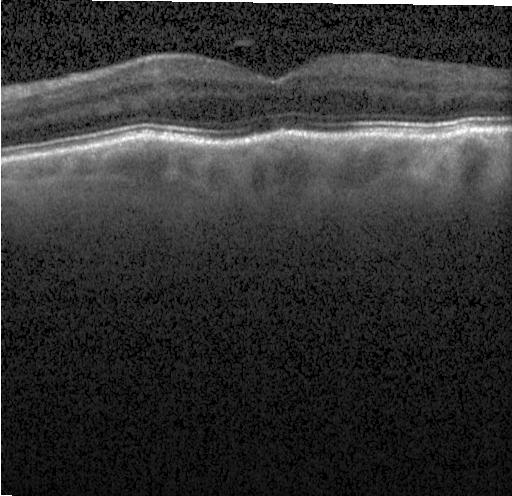

Finding: neither CNV, DME, nor drusen.